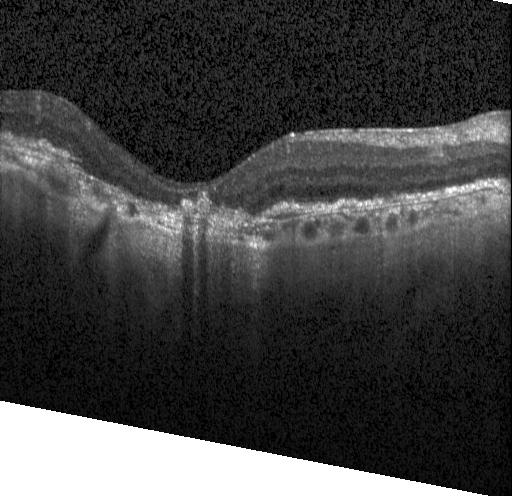
Macular scan. OCT line scan. Heidelberg Spectralis.
OCT finding: a choroidal neovascular membrane.